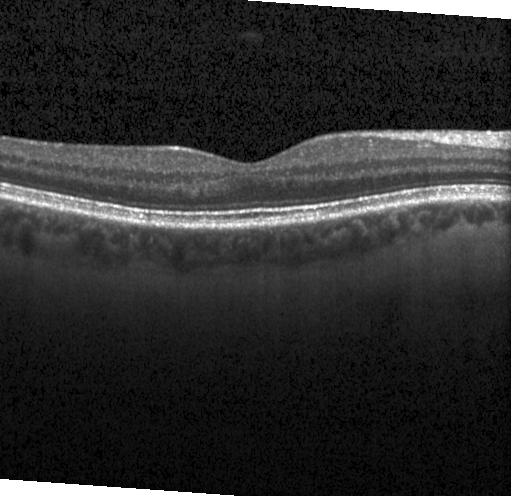

Optical coherence tomography scan. The scan shows no choroidal neovascularization, no diabetic macular edema, and no drusen.